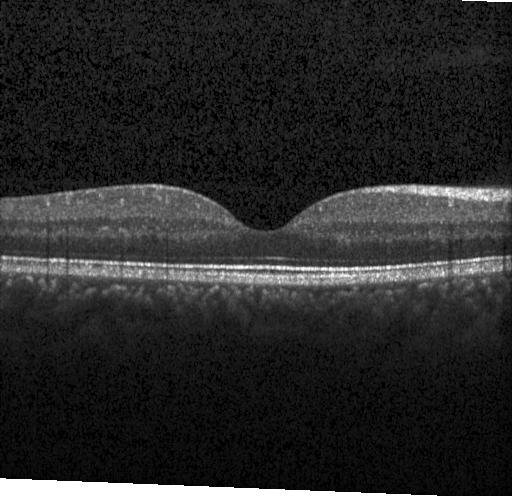

Optical coherence tomography scan.
This B-scan demonstrates no choroidal neovascularization, no diabetic macular edema, and no drusen.